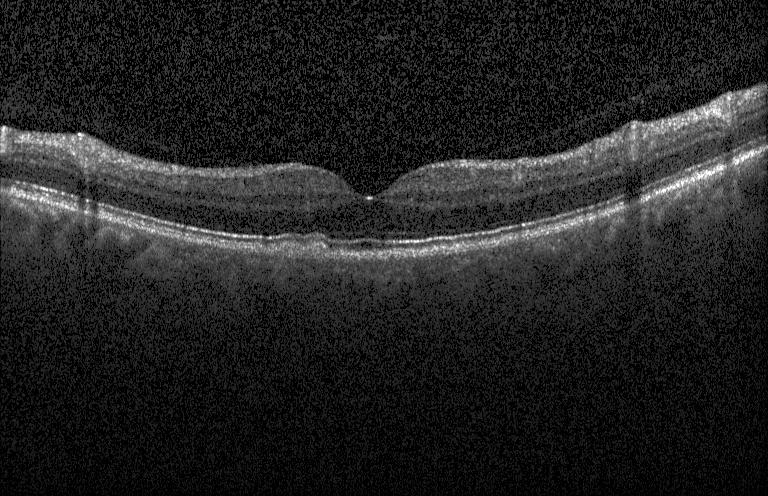

Retinal OCT cross-section. Finding: drusen.